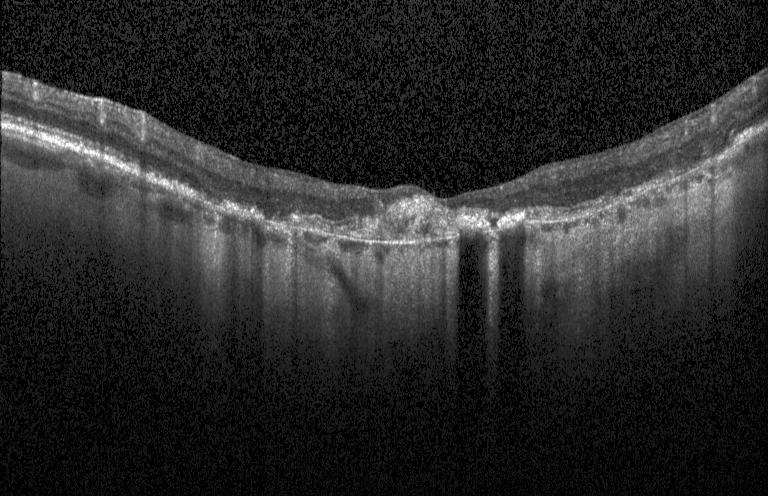

Optical coherence tomography scan · spectral-domain optical coherence tomography · acquired on a Heidelberg Spectralis — The scan shows a choroidal neovascular membrane.